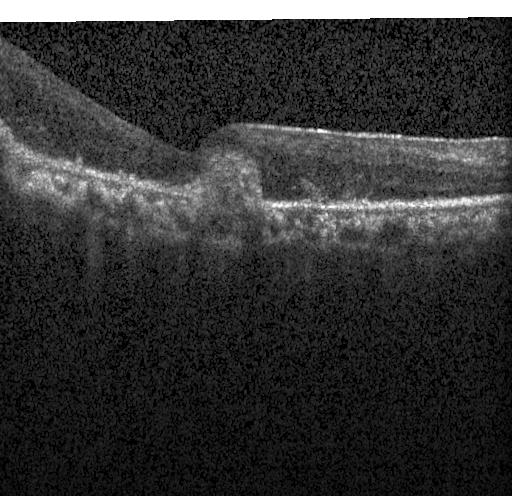

Optical coherence tomography B-scan
A choroidal neovascular membrane.